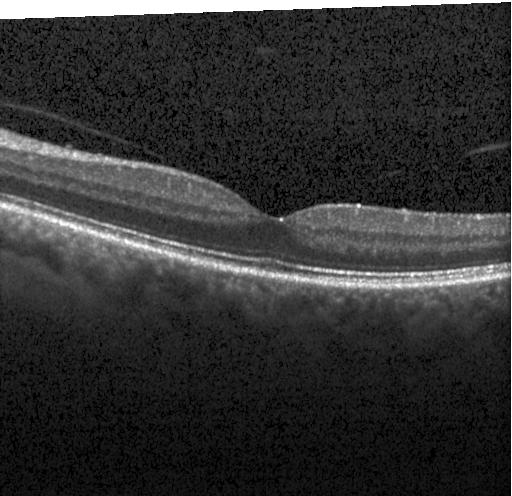 OCT B-scan showing no evidence of CNV, DME, or drusen.